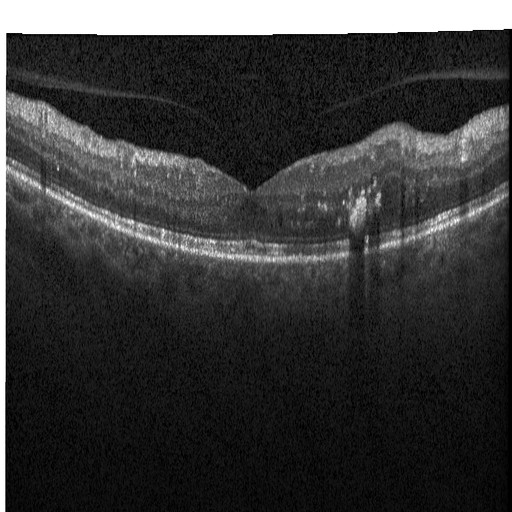 Impression: diabetic macular edema.